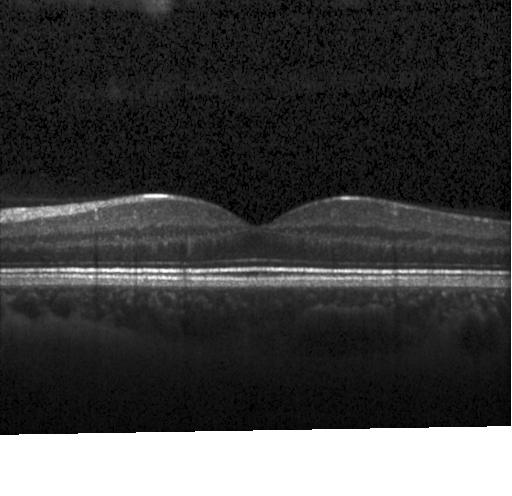
Centered on the fovea. Optical coherence tomography scan
The scan shows no choroidal neovascularization, diabetic macular edema, or drusen.